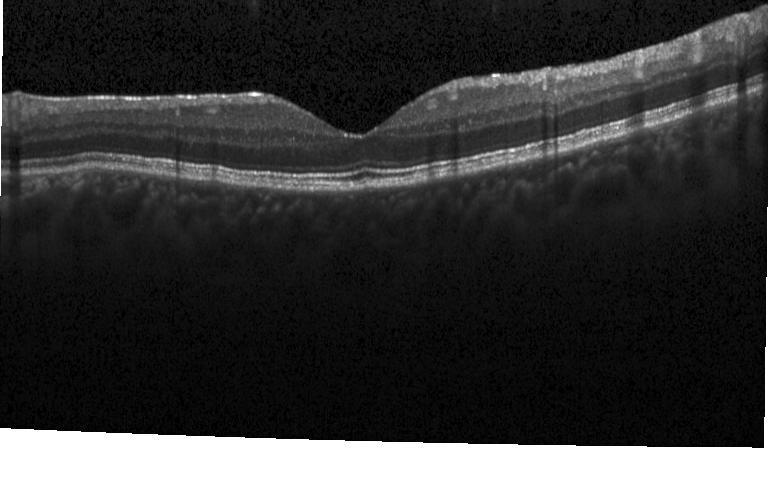
Spectral-domain optical coherence tomography; retinal OCT cross-section; Heidelberg Spectralis OCT system; fovea-centered — The scan shows no CNV, DME, or drusen.